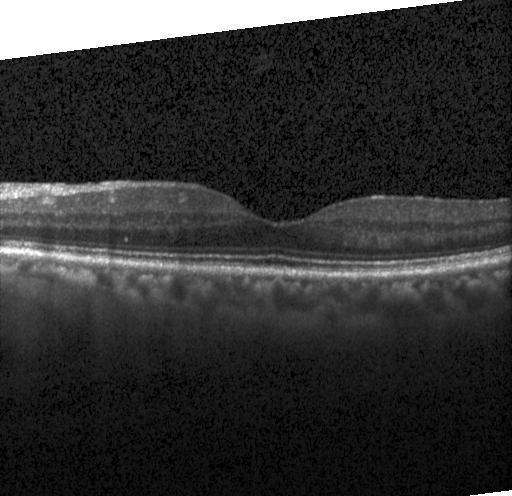
Retinal OCT cross-section · spectral-domain optical coherence tomography · fovea-centered
Macular OCT: no choroidal neovascularization, no diabetic macular edema, and no drusen.